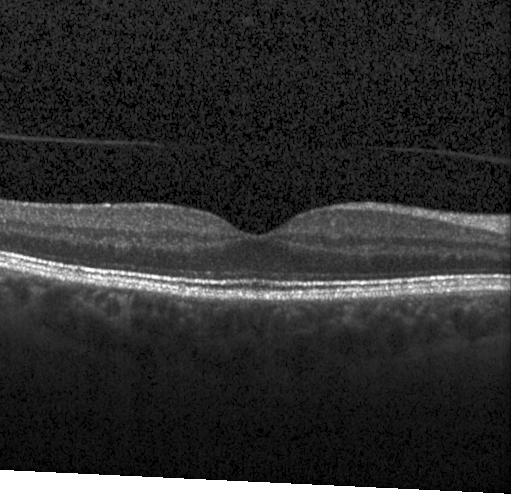
Fovea-centered; SD-OCT; optical coherence tomography scan. Finding: no CNV, no DME, and no drusen.